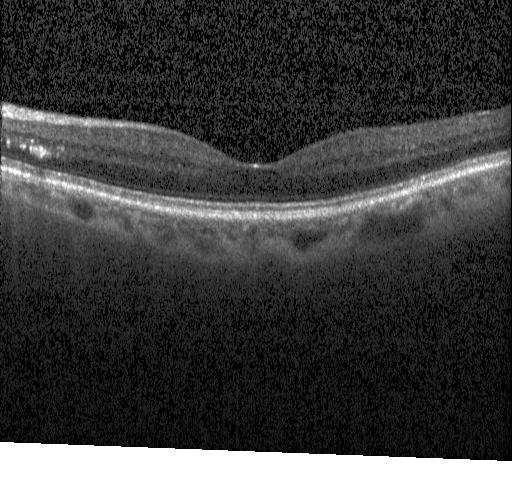

Retinal OCT cross-section.
Diagnosis: no CNV, no DME, and no drusen.